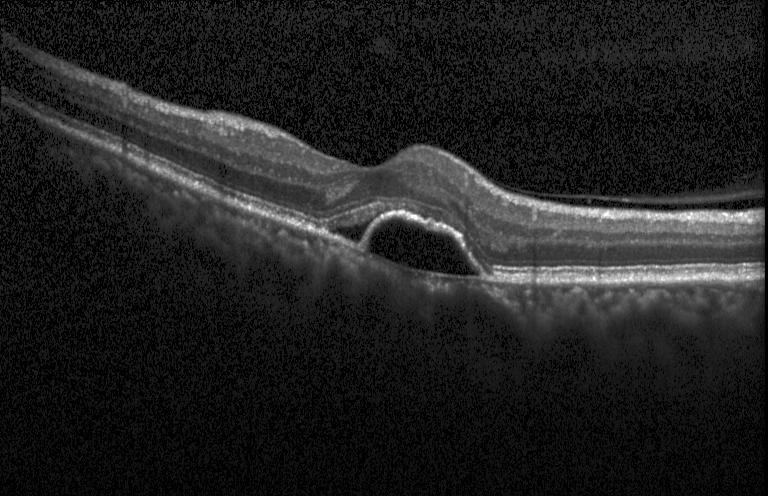 OCT B-scan.
Dx: CNV.